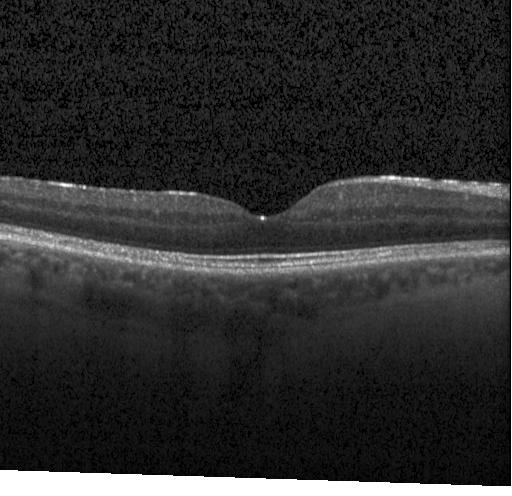 OCT B-scan.
Finding: neither choroidal neovascularization, diabetic macular edema, nor drusen.